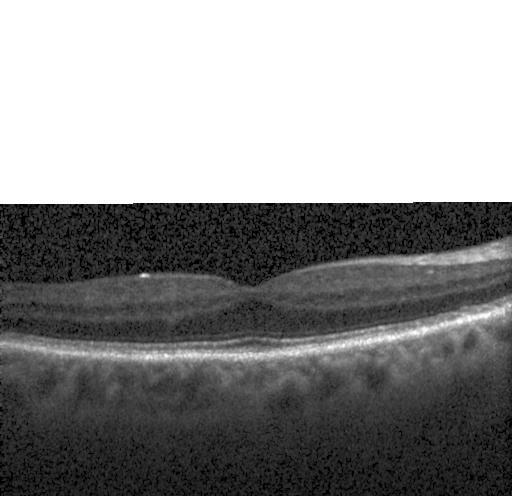
Horizontal scan through the fovea; spectral-domain optical coherence tomography; acquired on a Heidelberg Spectralis; OCT B-scan — Finding: no CNV, DME, or drusen.